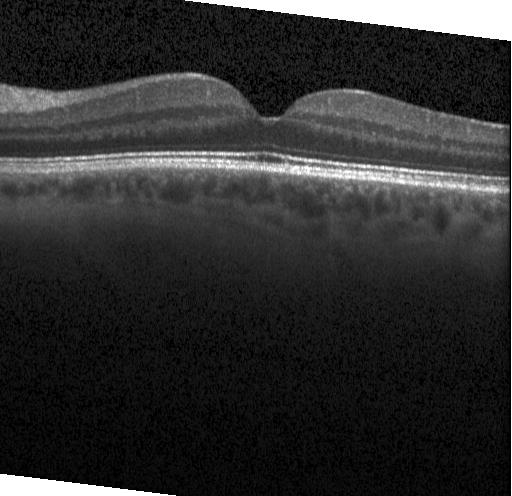
Optical coherence tomography scan · spectral-domain OCT · Heidelberg Spectralis. Diagnosis: no evidence of choroidal neovascularization, diabetic macular edema, or drusen.